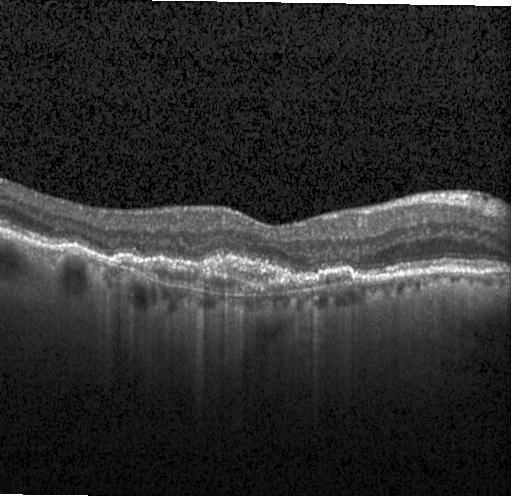
Finding: CNV.